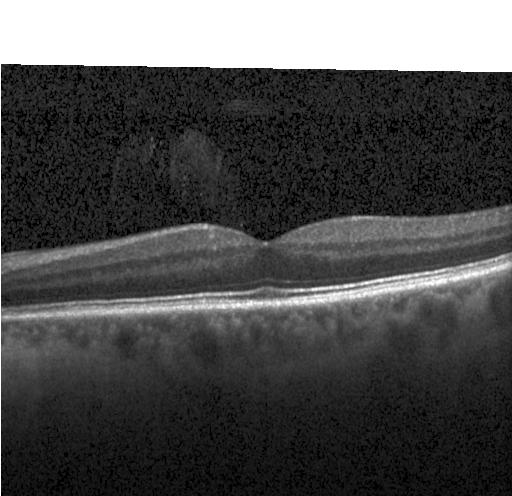 Optical coherence tomography scan · horizontal scan through the fovea · spectral-domain optical coherence tomography
This B-scan demonstrates no choroidal neovascularization, diabetic macular edema, or drusen.